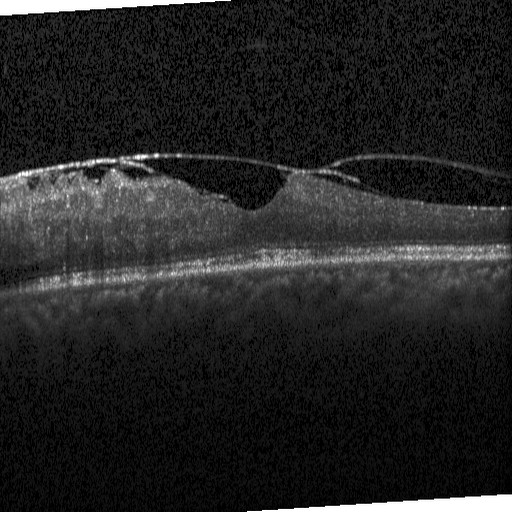
Instrument: Heidelberg Spectralis · horizontal scan through the fovea · retinal OCT cross-section. Finding: DME.